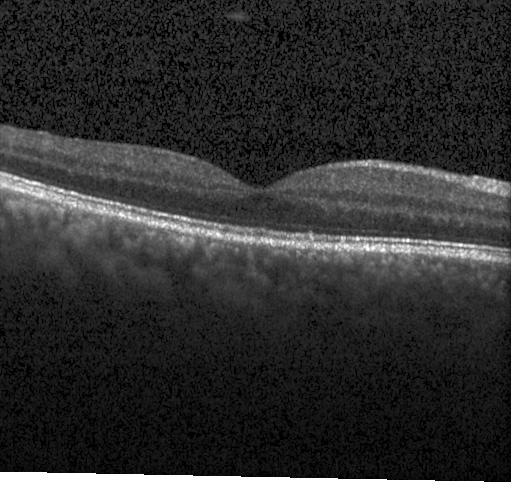
Spectral-domain optical coherence tomography; through the macula; Heidelberg Spectralis; optical coherence tomography B-scan
Impression: no choroidal neovascularization, no diabetic macular edema, and no drusen.